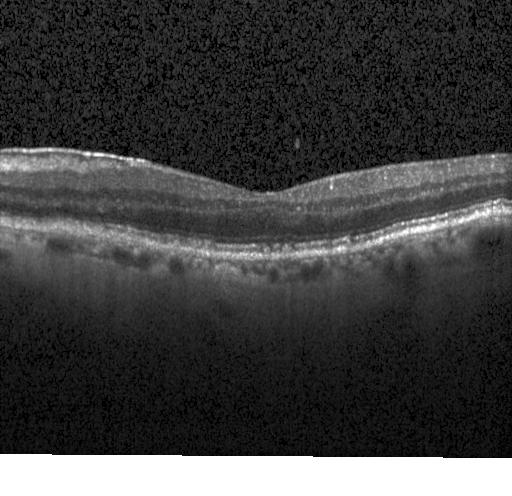 Optical coherence tomography scan, SD-OCT — Assessment: drusen.